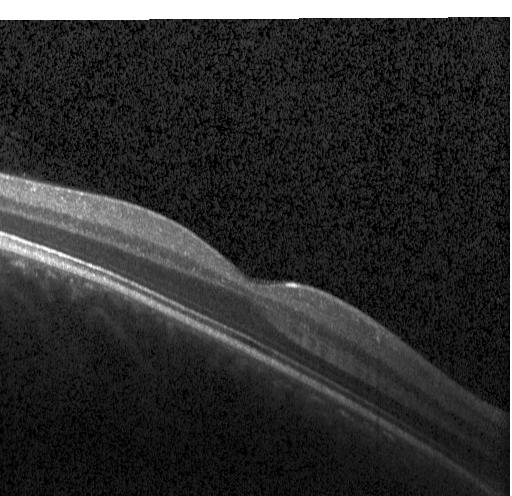 OCT line scan. Macular OCT: neither CNV, DME, nor drusen.